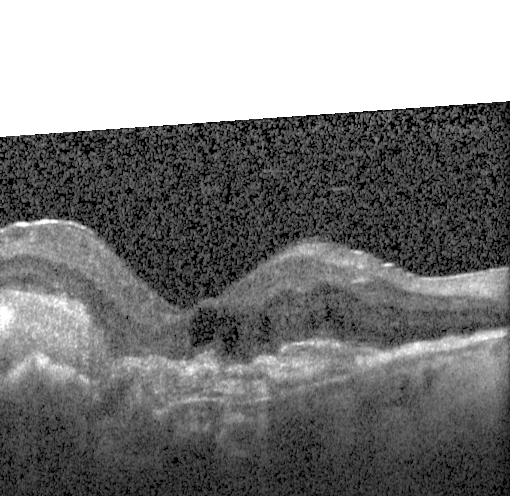
OCT scan showing choroidal neovascularization (CNV).